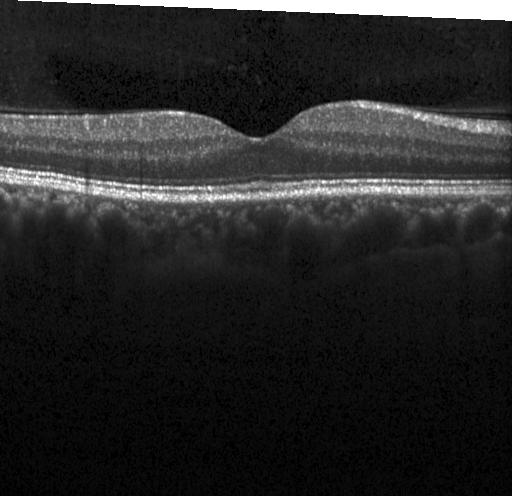
OCT scan showing no CNV, DME, or drusen.